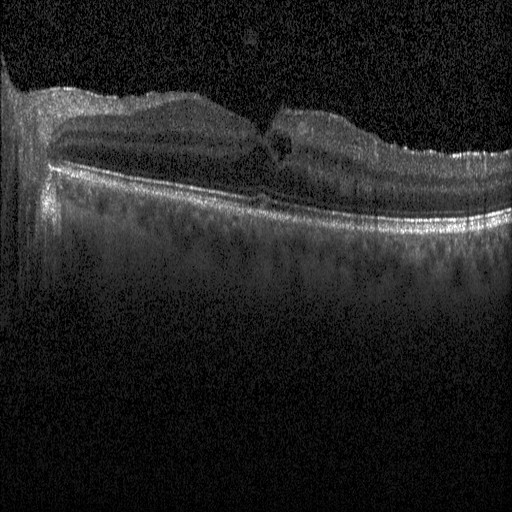

Macular OCT demonstrating diabetic macular edema (DME).